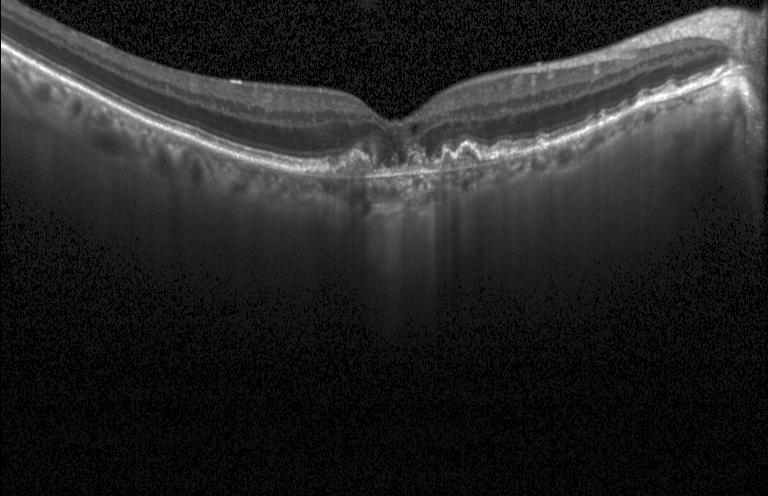 OCT B-scan, spectral-domain OCT, centered on the fovea, acquired on a Heidelberg Spectralis.
A choroidal neovascular membrane.